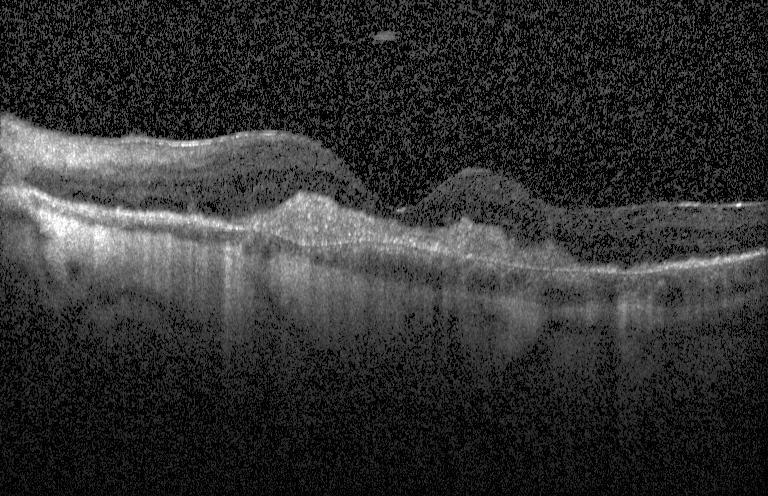

Retinal OCT cross-section.
Impression: choroidal neovascularization.